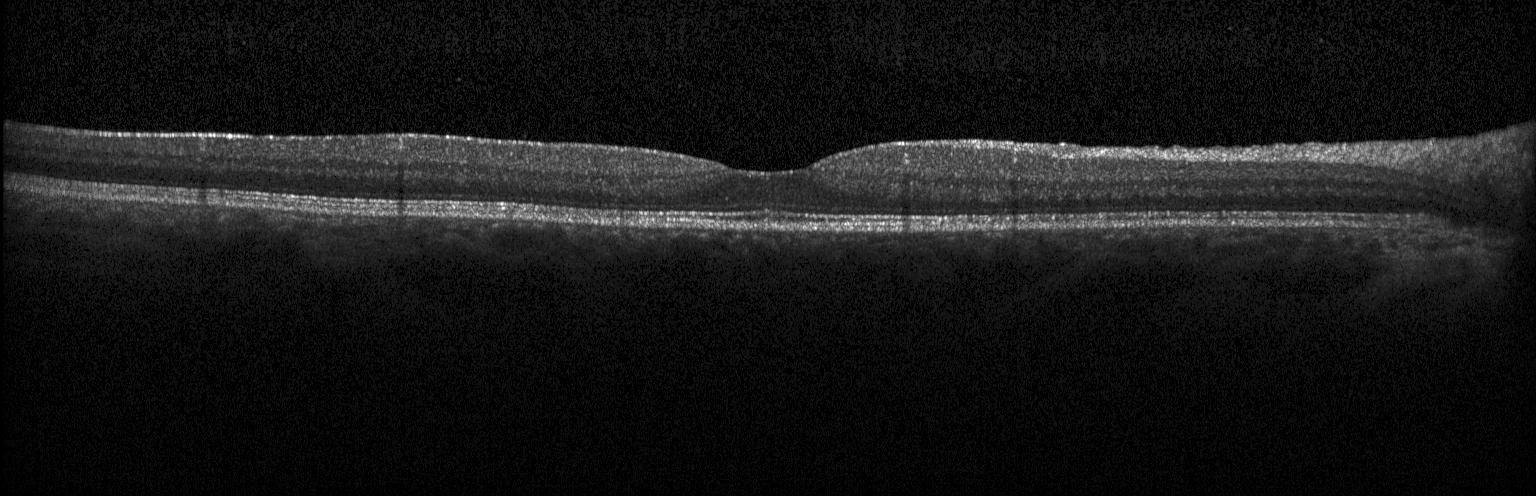
Retinal OCT cross-section.
Impression: no evidence of choroidal neovascularization, diabetic macular edema, or drusen.